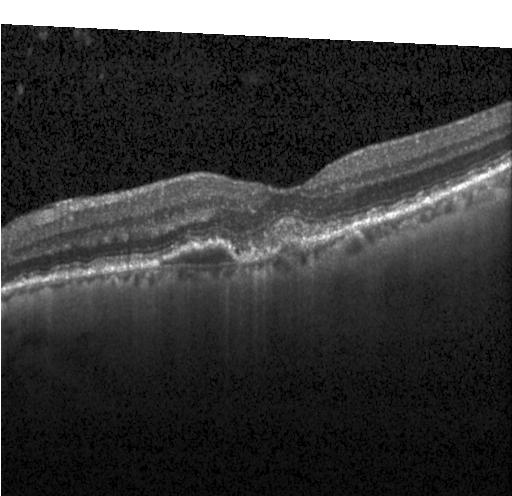 Finding: CNV.